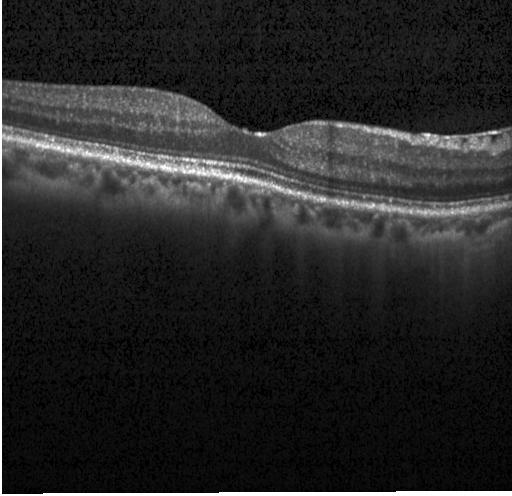

Spectral-domain OCT; centered on the fovea; retinal OCT B-scan; Heidelberg Spectralis — Finding: neither choroidal neovascularization, diabetic macular edema, nor drusen.